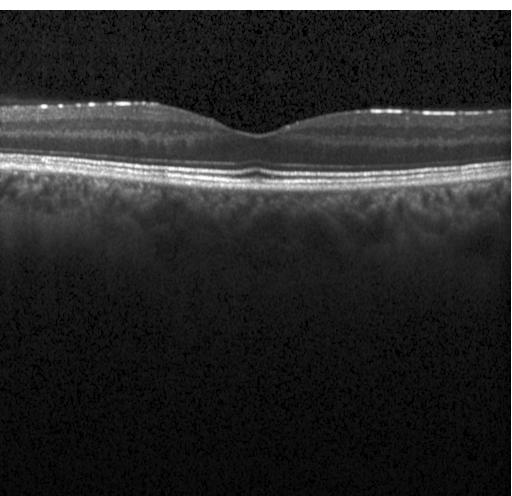 Retinal OCT B-scan — Assessment: no evidence of CNV, DME, or drusen.